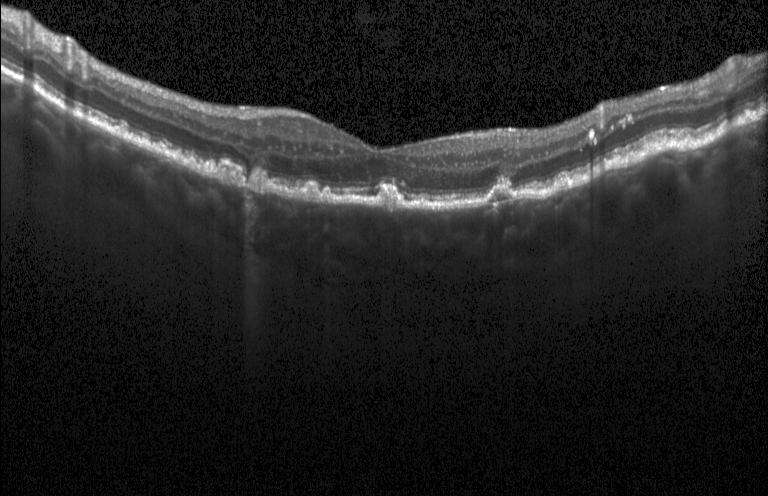

Macular OCT: drusen.